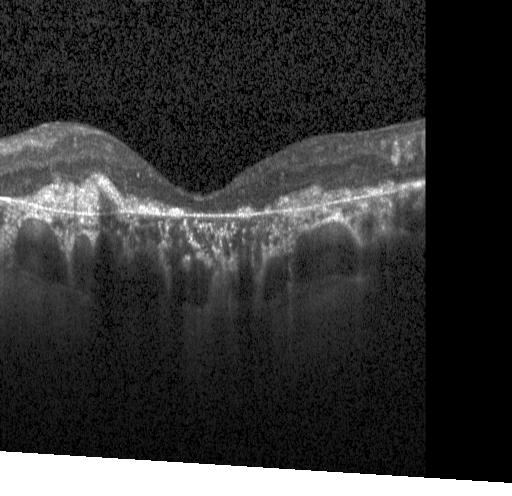

Through the macula, optical coherence tomography B-scan, spectral-domain OCT. Diagnosis: a choroidal neovascular membrane.